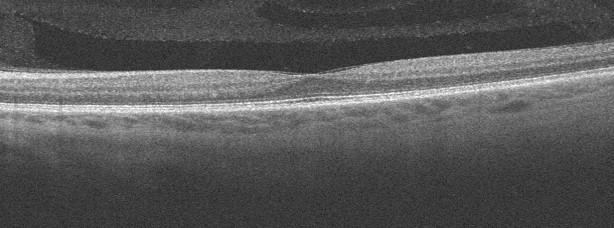

Fovea-centered · acquired on an Optovue Avanti RTVue XR · retinal OCT B-scan. Finding: no evidence of AMD, DME, ERM, RAO, RVO, or VID.